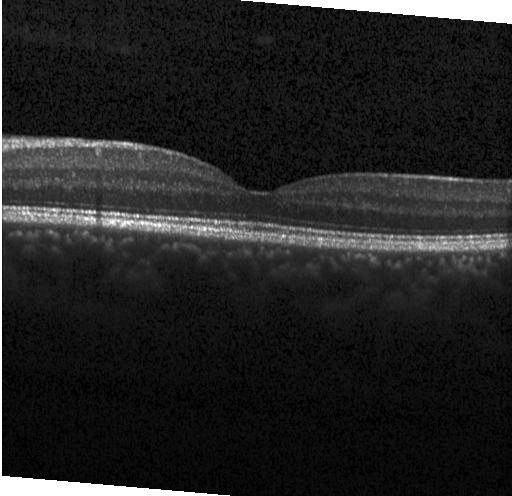

OCT line scan. Spectral-domain optical coherence tomography — Diagnosis: no CNV, no DME, and no drusen.